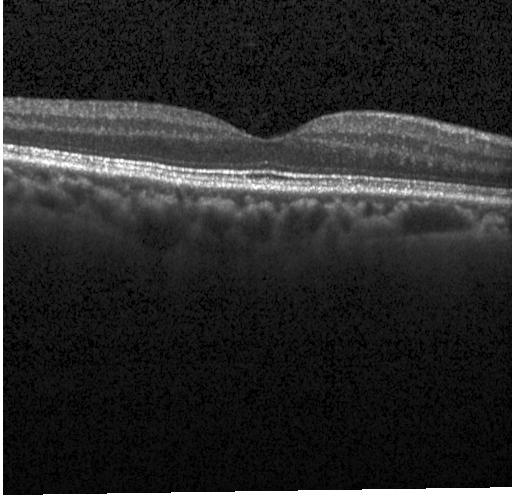 Optical coherence tomography scan. Heidelberg Spectralis OCT system. Horizontal scan through the fovea. SD-OCT
Impression: no choroidal neovascularization, no diabetic macular edema, and no drusen.